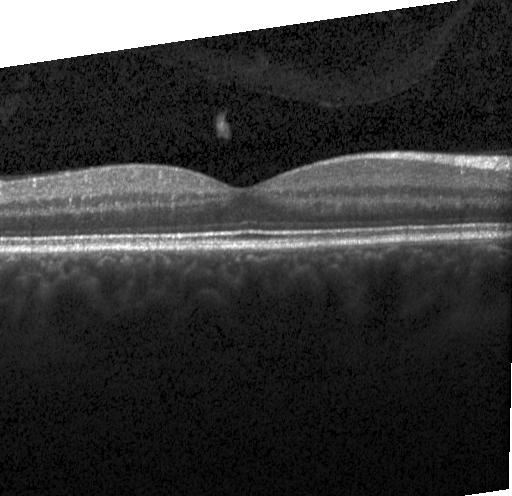
SD-OCT, optical coherence tomography scan, fovea-centered, instrument: Heidelberg Spectralis.
Impression: no evidence of CNV, DME, or drusen.